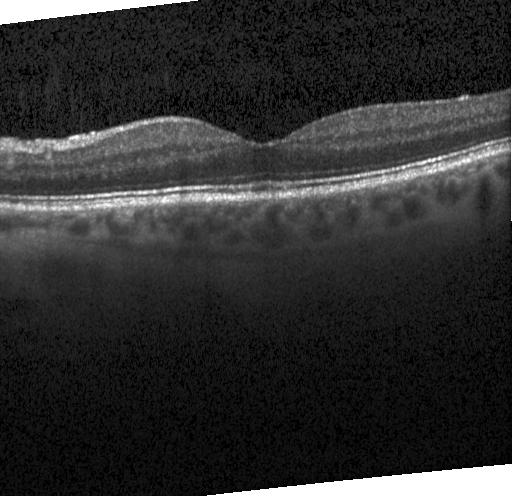
Diagnosis: no evidence of CNV, DME, or drusen.